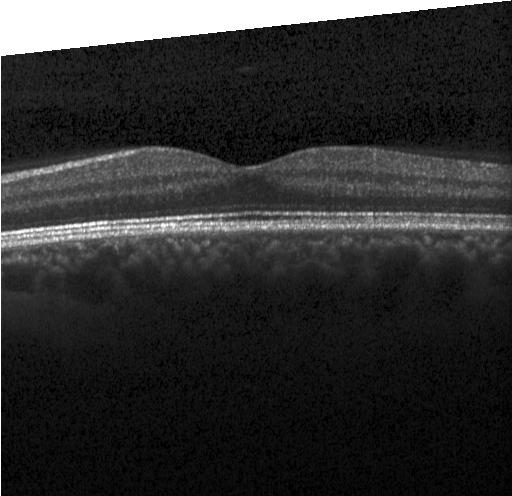
Optical coherence tomography B-scan
Finding: neither choroidal neovascularization, diabetic macular edema, nor drusen.